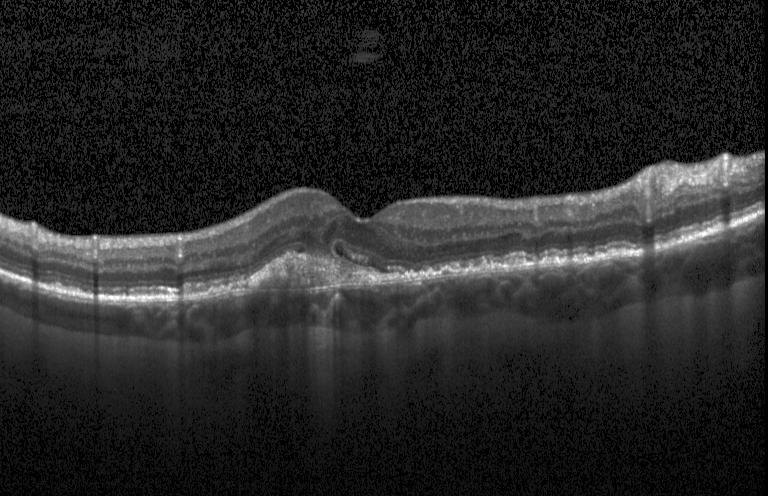
Retinal OCT B-scan — Choroidal neovascularization (CNV).